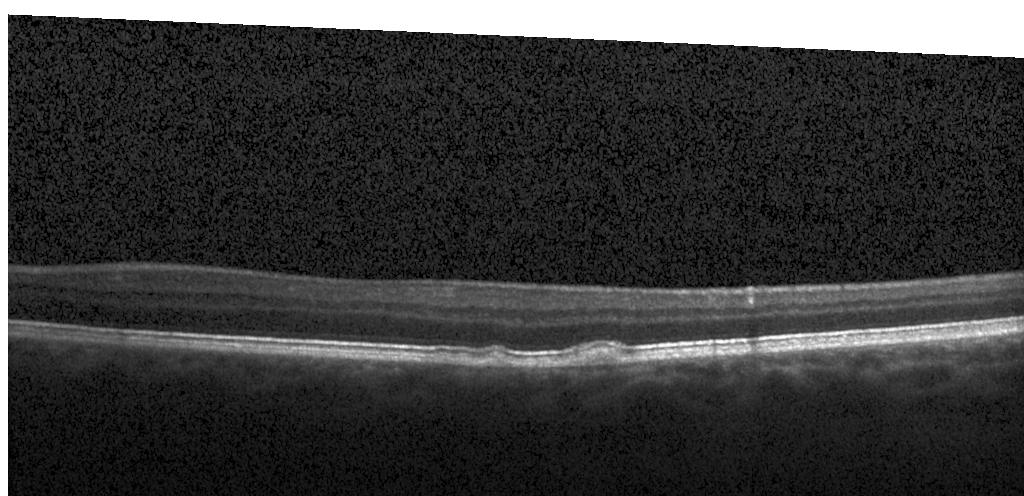

Macular OCT demonstrating drusen.